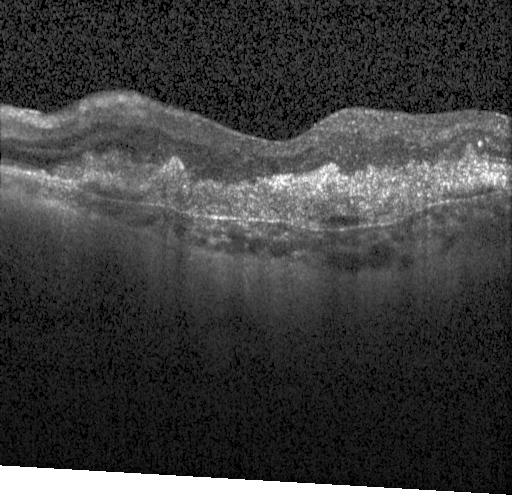

OCT line scan. This B-scan demonstrates choroidal neovascularization.